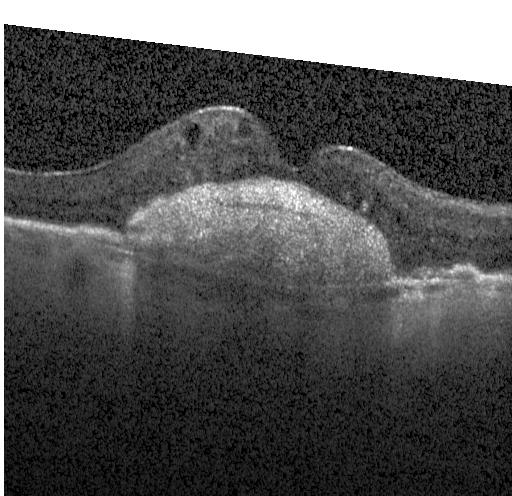
Macular OCT demonstrating a choroidal neovascular membrane.